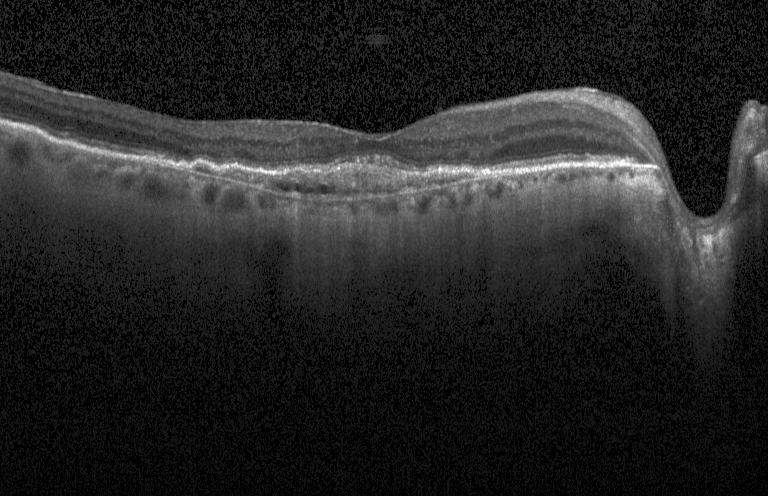 Heidelberg Spectralis OCT system, optical coherence tomography B-scan.
Diagnosis: a choroidal neovascular membrane.